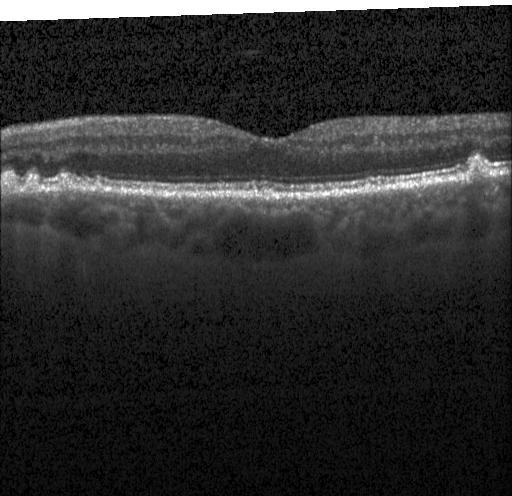 Macular OCT demonstrating multiple drusen.